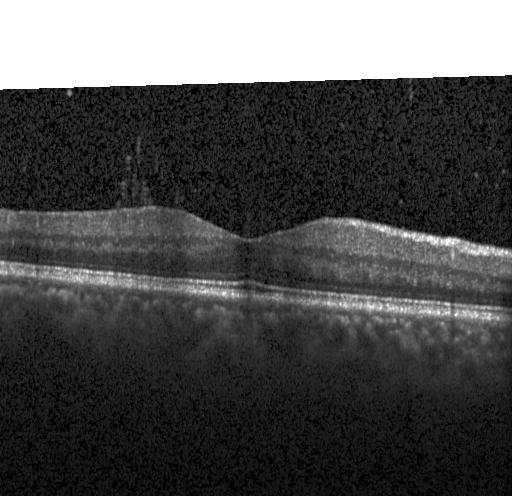 OCT line scan; Heidelberg Spectralis; spectral-domain OCT — The scan shows neither choroidal neovascularization, diabetic macular edema, nor drusen.